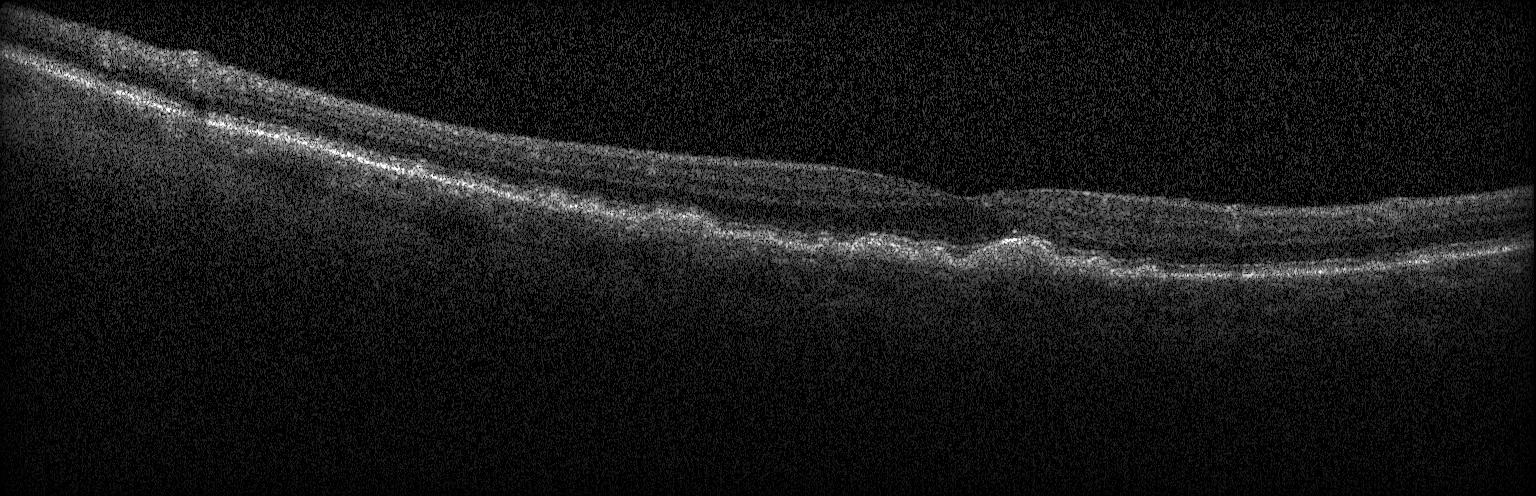
Fovea-centered, acquired on a Heidelberg Spectralis, optical coherence tomography scan. Diagnosis: multiple drusen.